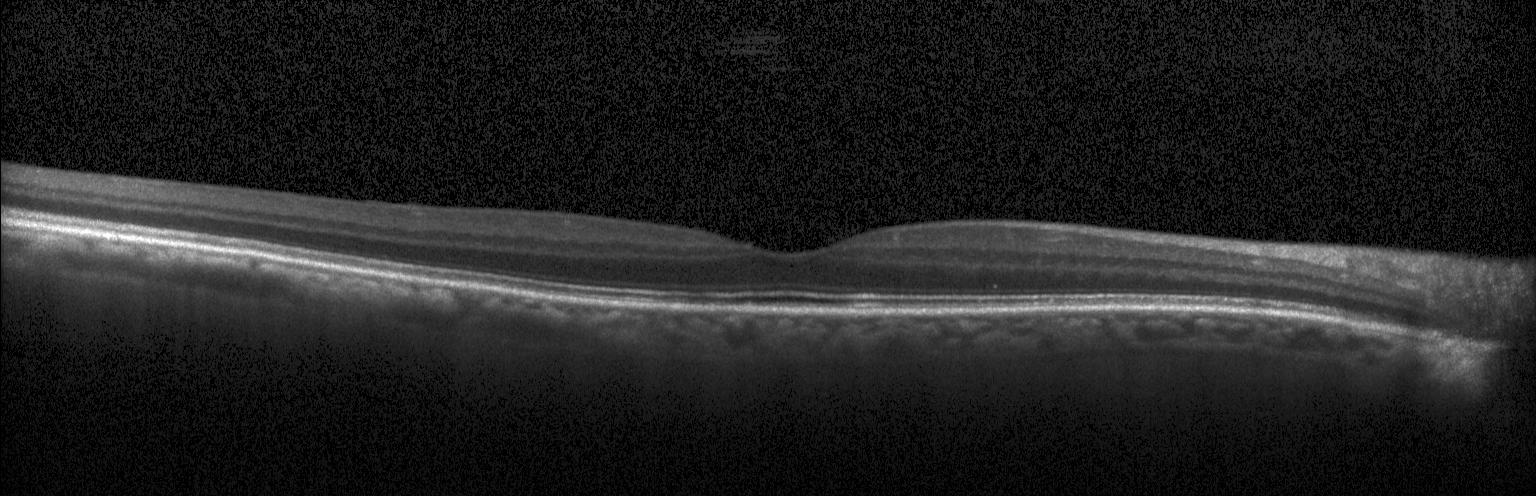
Retinal OCT cross-section, Heidelberg Spectralis OCT system.
Macular OCT: no choroidal neovascularization, no diabetic macular edema, and no drusen.